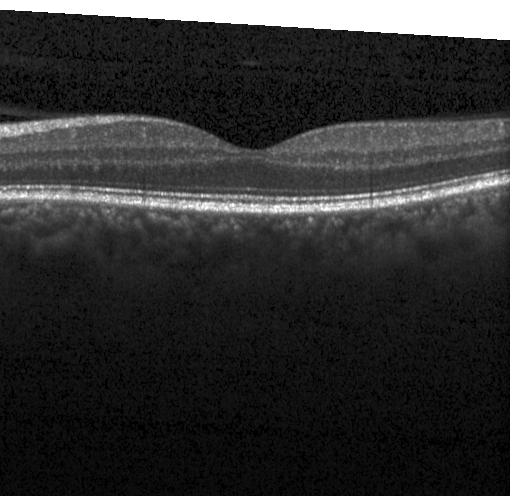

Spectral-domain OCT B-scan: no CNV, no DME, and no drusen.